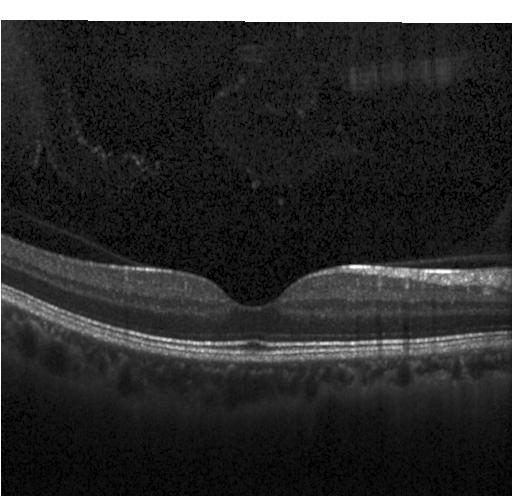 Finding: no evidence of choroidal neovascularization, diabetic macular edema, or drusen.